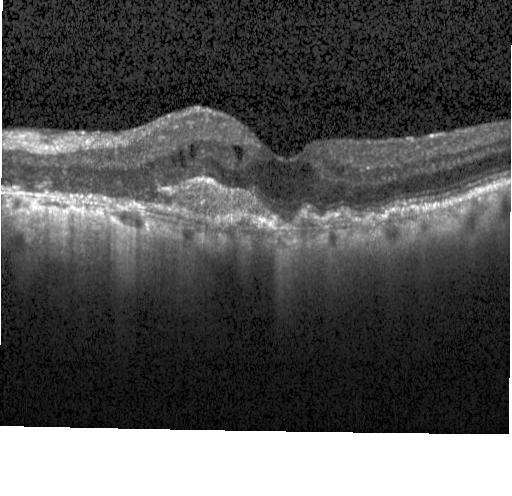

Assessment: a choroidal neovascular membrane.